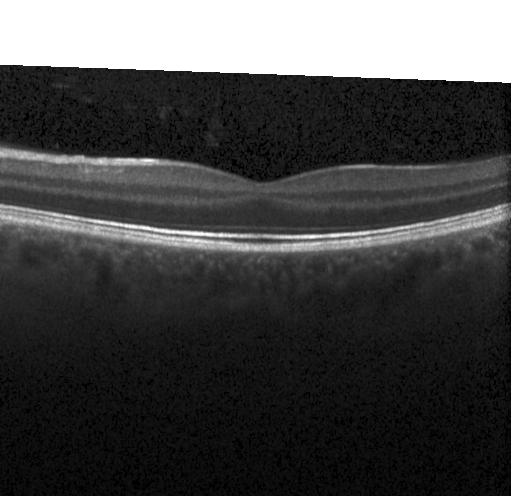 Impression: no choroidal neovascularization, no diabetic macular edema, and no drusen.